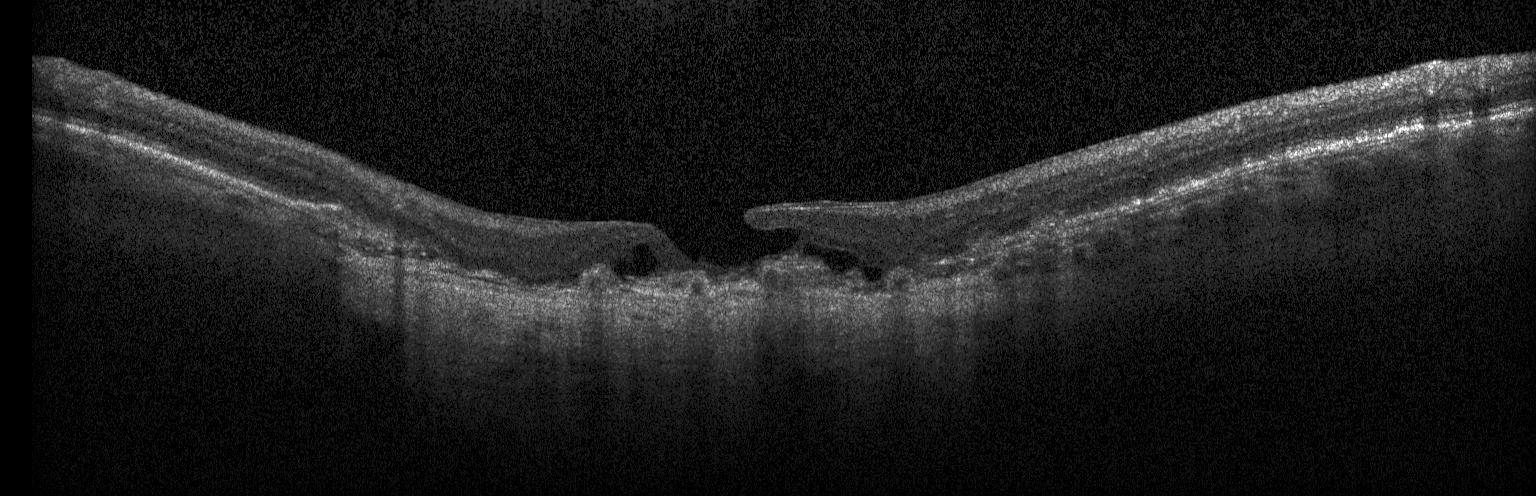 OCT B-scan.
This B-scan demonstrates choroidal neovascularization.